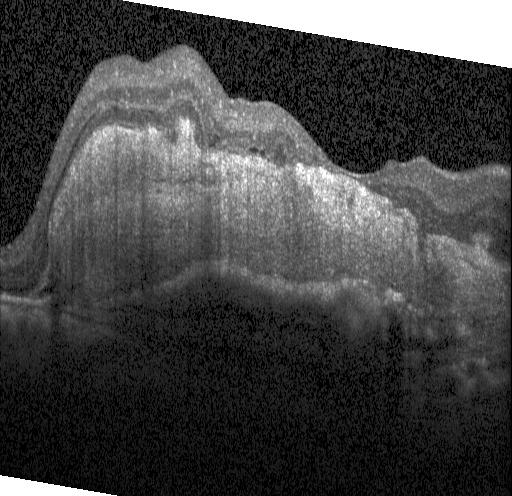

Heidelberg Spectralis OCT system; optical coherence tomography B-scan; centered on the fovea — The scan shows CNV.